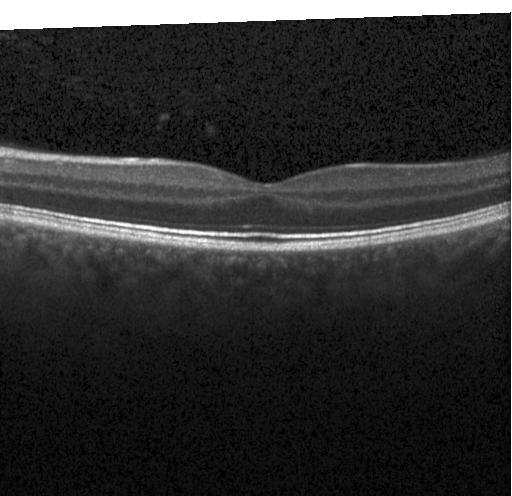

OCT scan showing no choroidal neovascularization, diabetic macular edema, or drusen.